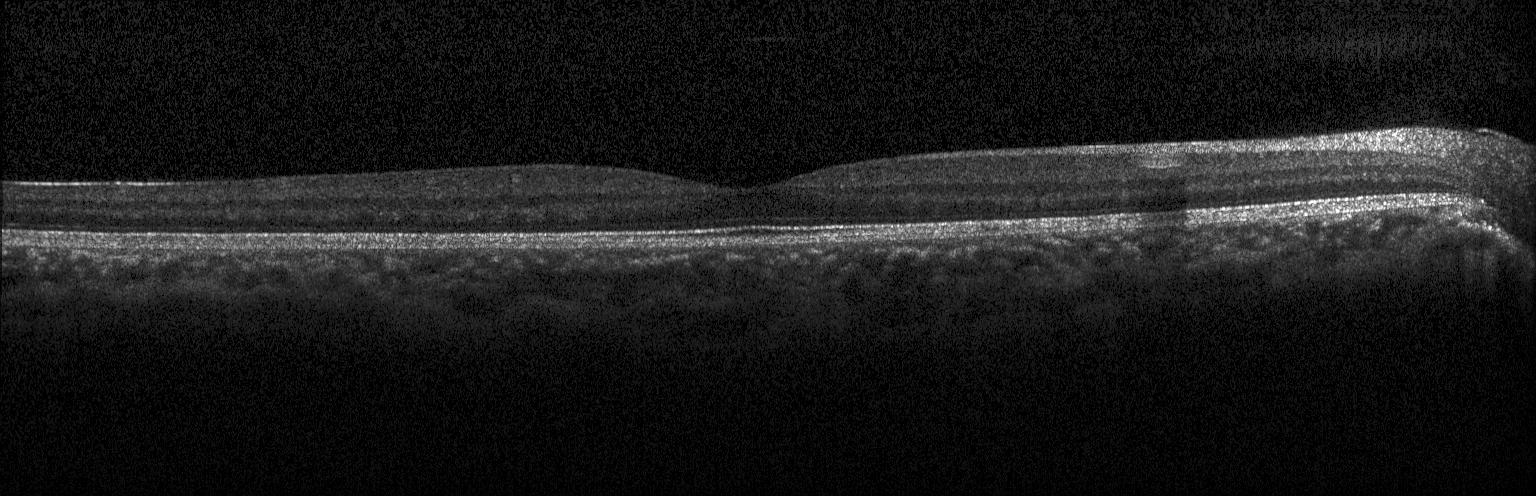
OCT B-scan showing no CNV, DME, or drusen.